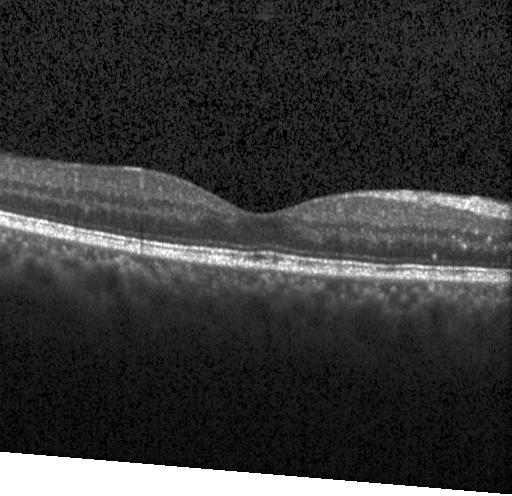

OCT line scan, fovea-centered, spectral-domain OCT, Heidelberg Spectralis OCT system.
No evidence of choroidal neovascularization, diabetic macular edema, or drusen.